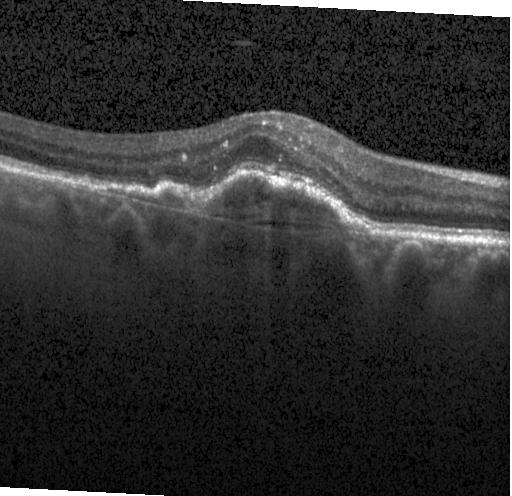 Spectral-domain OCT, OCT B-scan — Assessment: choroidal neovascularization (CNV).